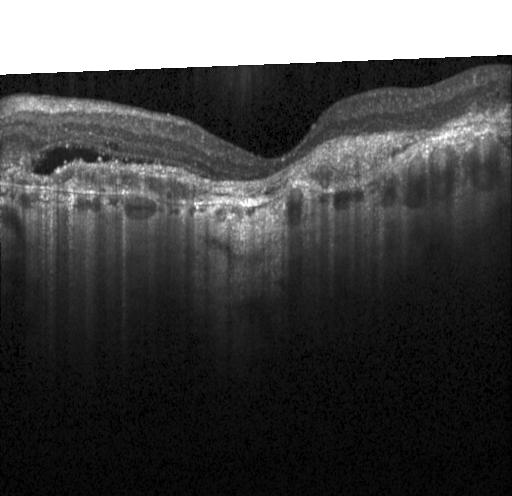

Assessment: a choroidal neovascular membrane.